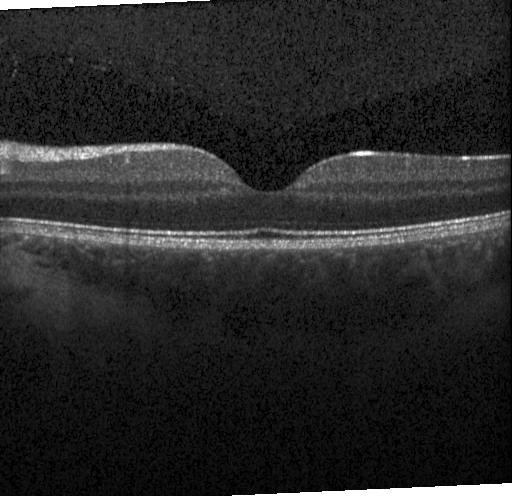 OCT line scan
No evidence of choroidal neovascularization, diabetic macular edema, or drusen.